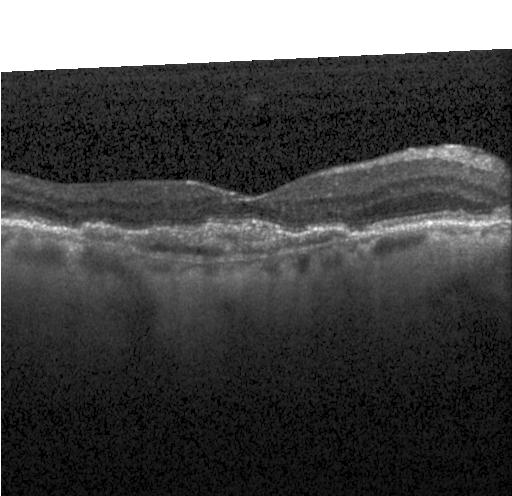

Diagnosis: choroidal neovascularization (CNV).